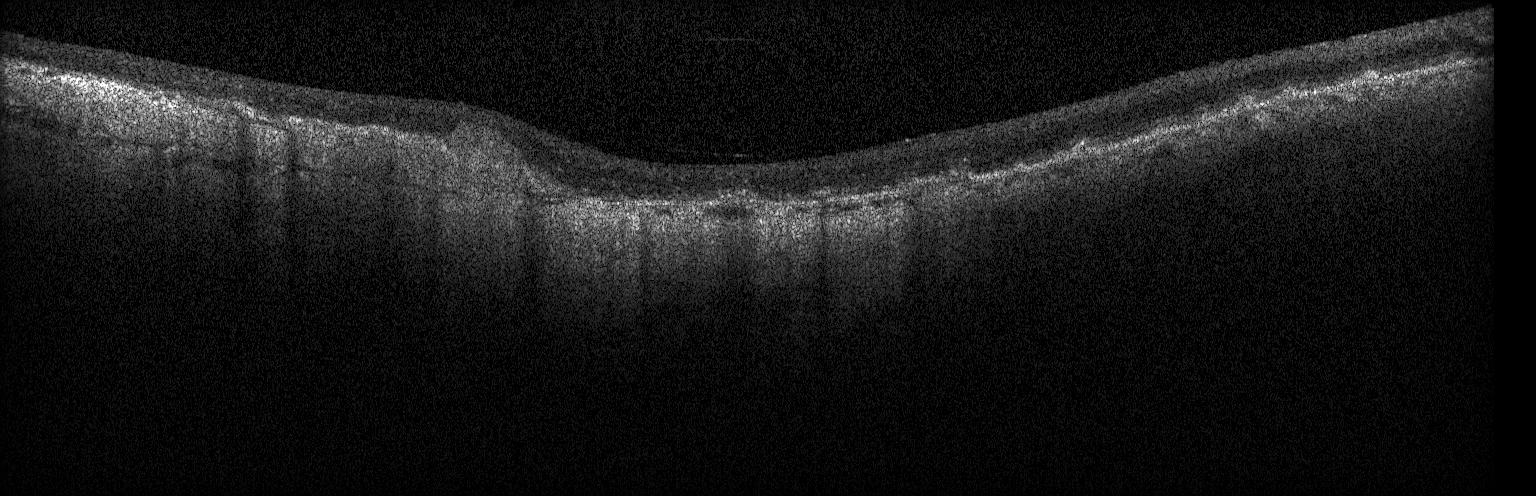

OCT B-scan; macular scan. Impression: CNV.